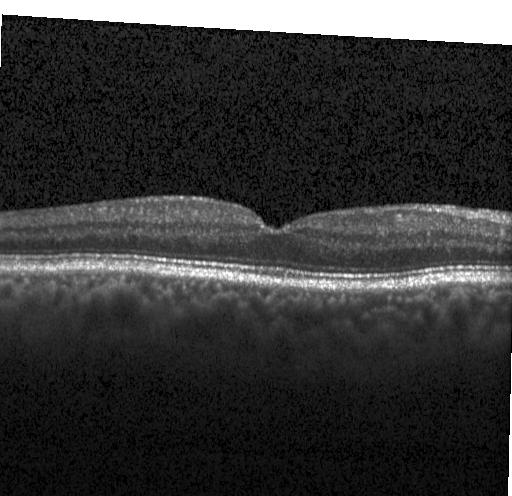
OCT scan showing no CNV, DME, or drusen.